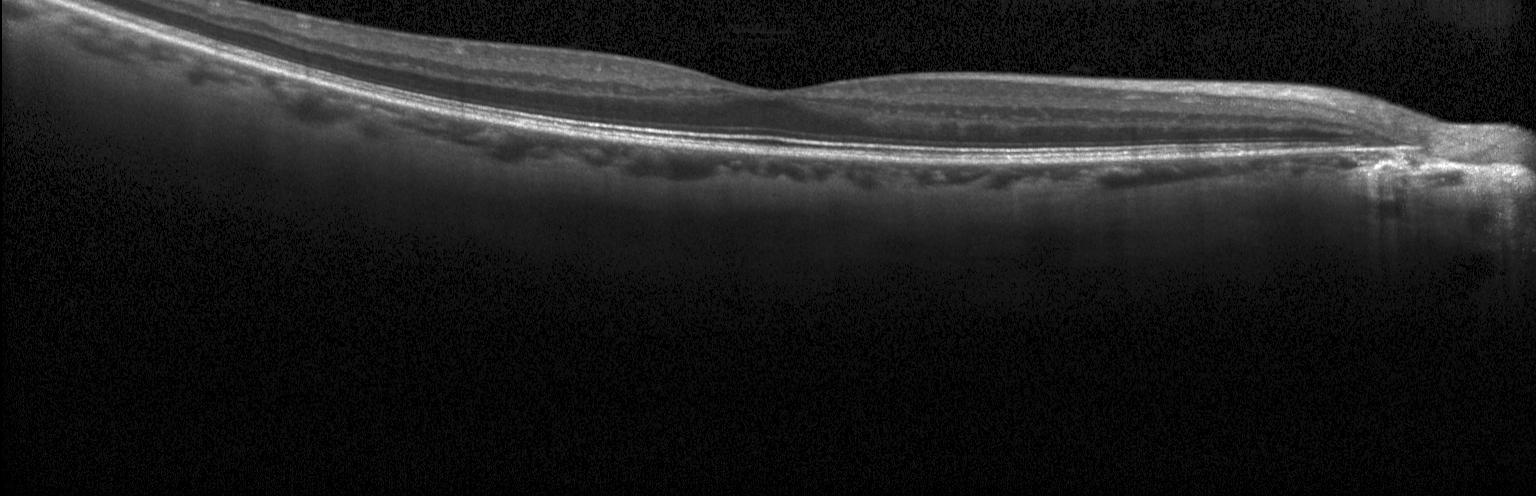 The scan shows no CNV, no DME, and no drusen.